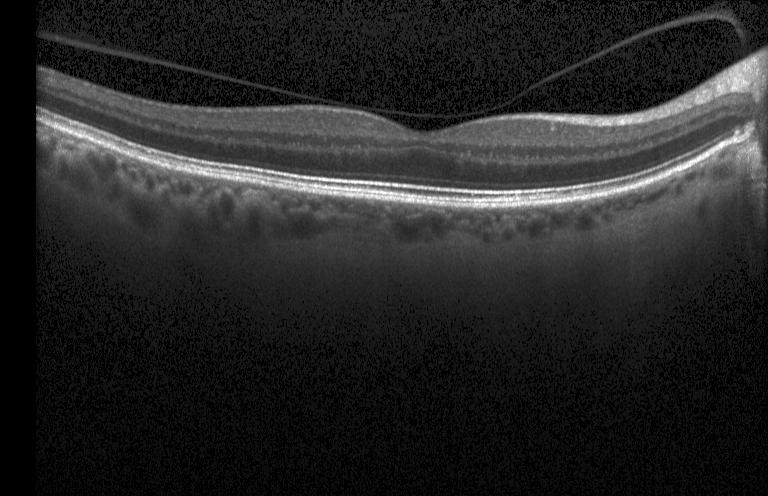
OCT line scan; Heidelberg Spectralis OCT system; macular scan; SD-OCT
Diagnosis: no choroidal neovascularization, no diabetic macular edema, and no drusen.